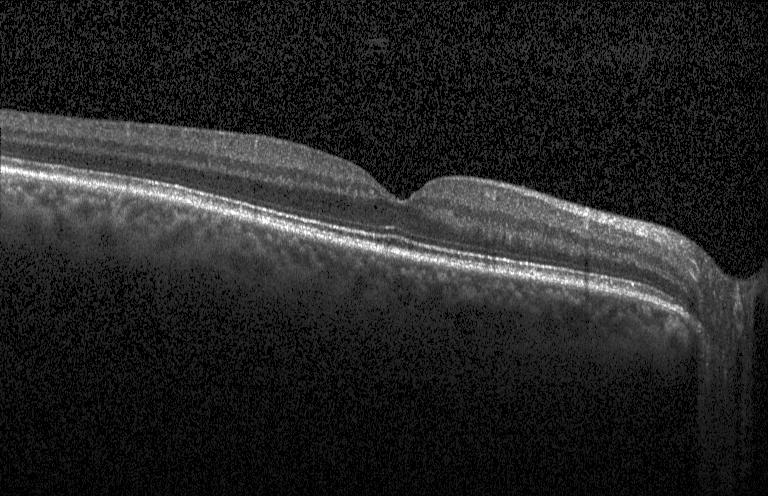

Optical coherence tomography B-scan. Impression: no evidence of choroidal neovascularization, diabetic macular edema, or drusen.